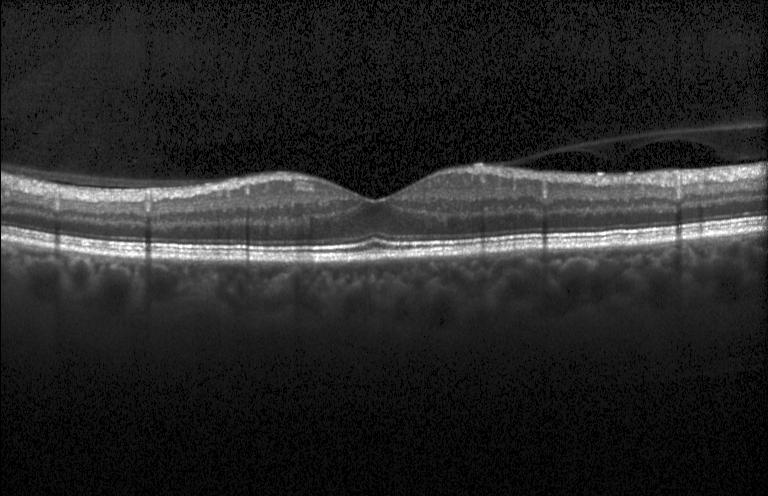 No evidence of choroidal neovascularization, diabetic macular edema, or drusen.